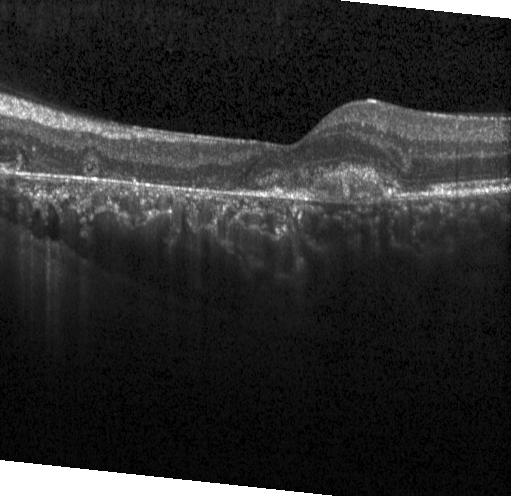

OCT line scan · SD-OCT · centered on the fovea — Finding: choroidal neovascularization (CNV).